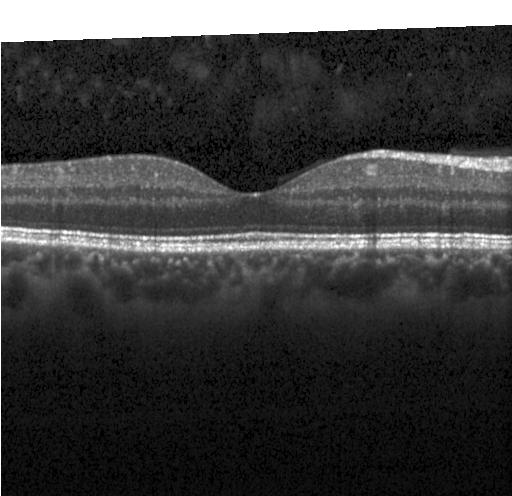

OCT B-scan · Heidelberg Spectralis OCT system — Finding: no CNV, DME, or drusen.